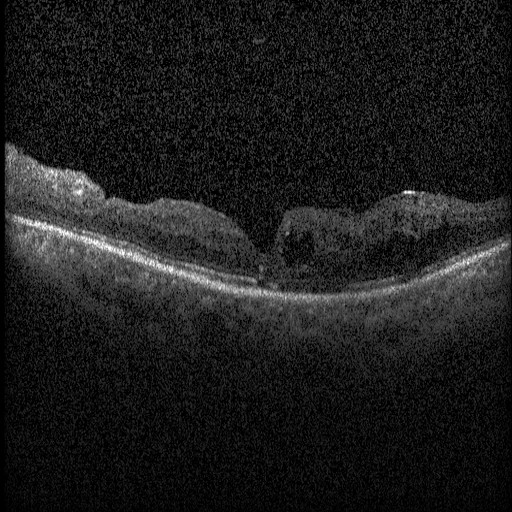
OCT line scan — Dx: diabetic macular edema.